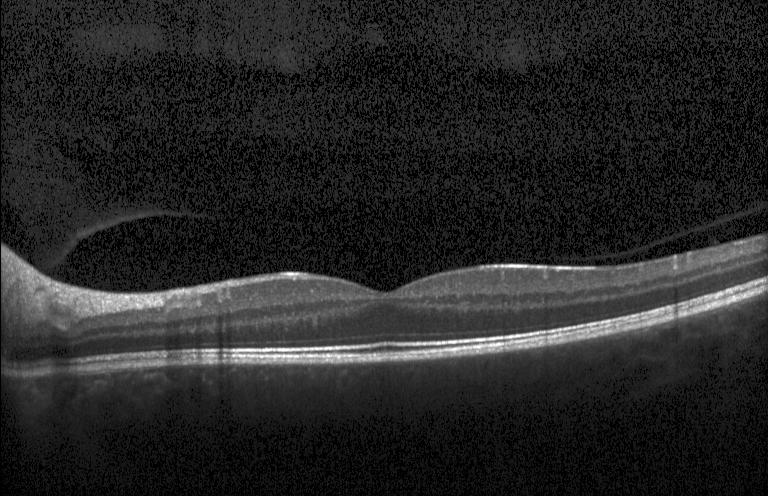
Optical coherence tomography scan. Horizontal scan through the fovea — Finding: no evidence of CNV, DME, or drusen.